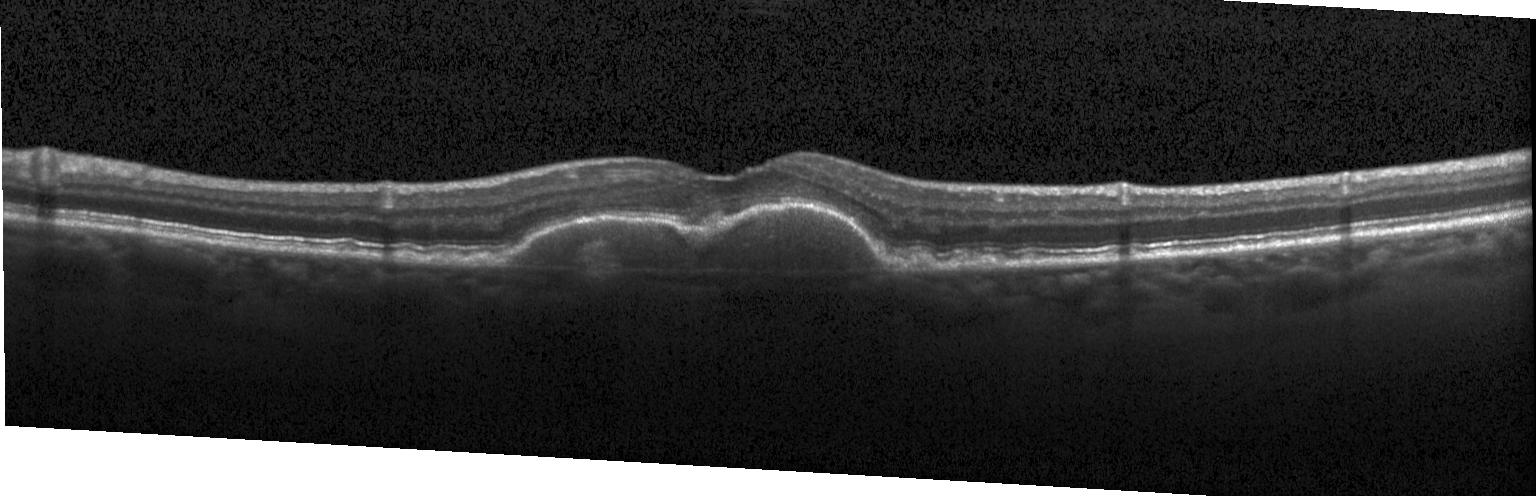

CNV.